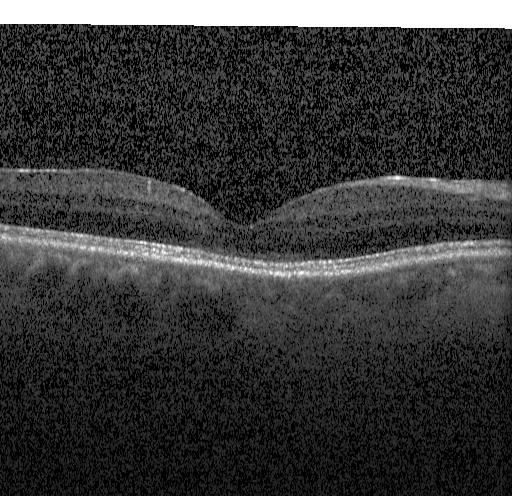
Dx: no CNV, DME, or drusen.